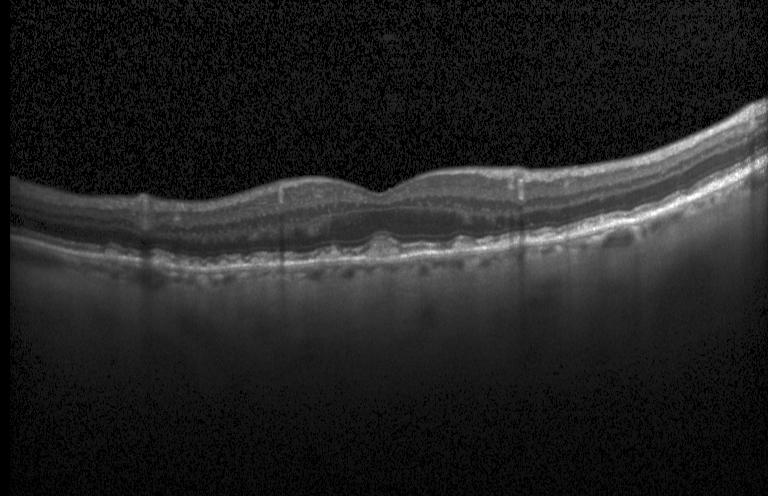 Macular scan, retinal OCT B-scan, spectral-domain optical coherence tomography. Diagnosis: sub-RPE drusenoid deposits.